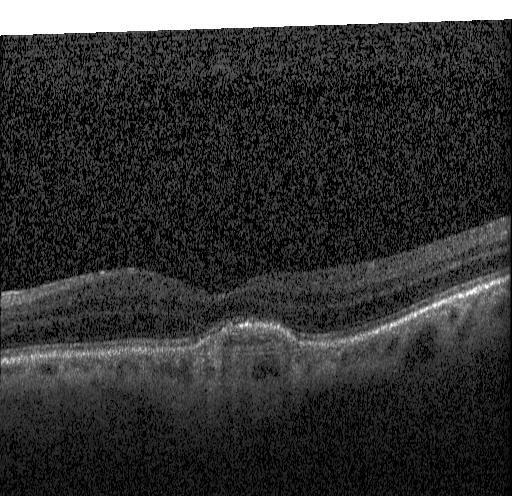
Heidelberg Spectralis OCT system, optical coherence tomography B-scan — Impression: a choroidal neovascular membrane.